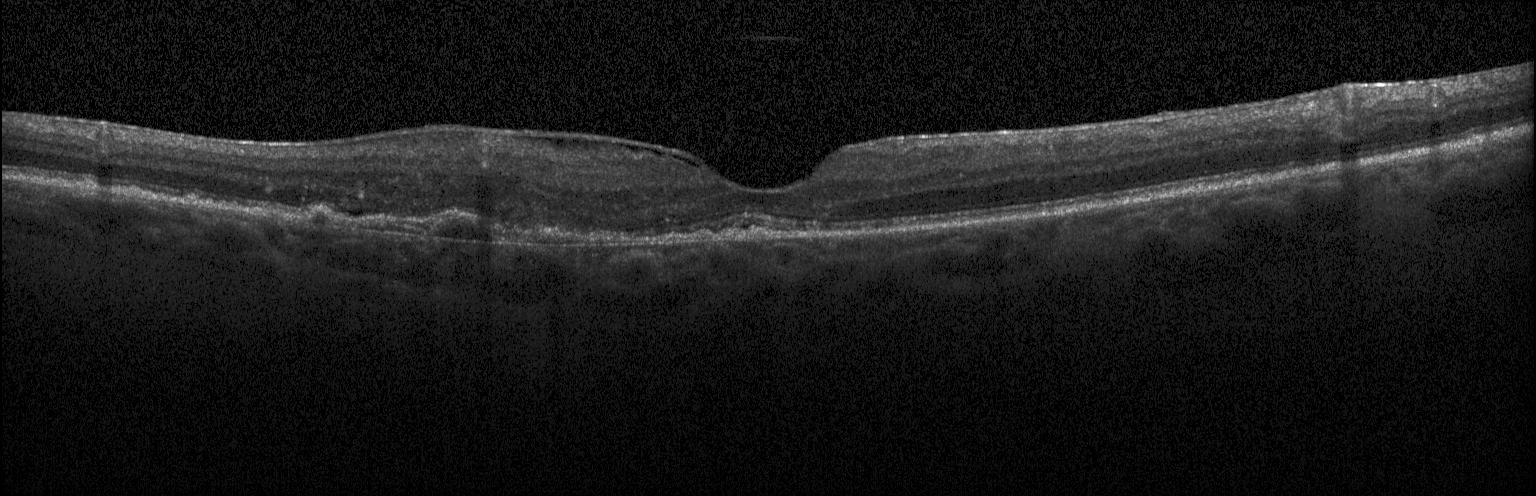
Heidelberg Spectralis OCT system, optical coherence tomography B-scan — A choroidal neovascular membrane.